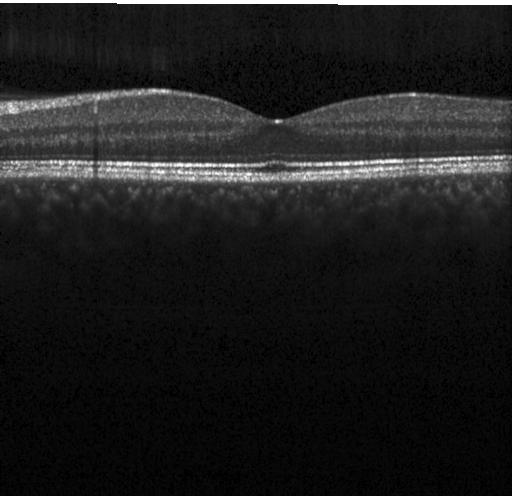 Optical coherence tomography scan. Diagnosis: no CNV, no DME, and no drusen.